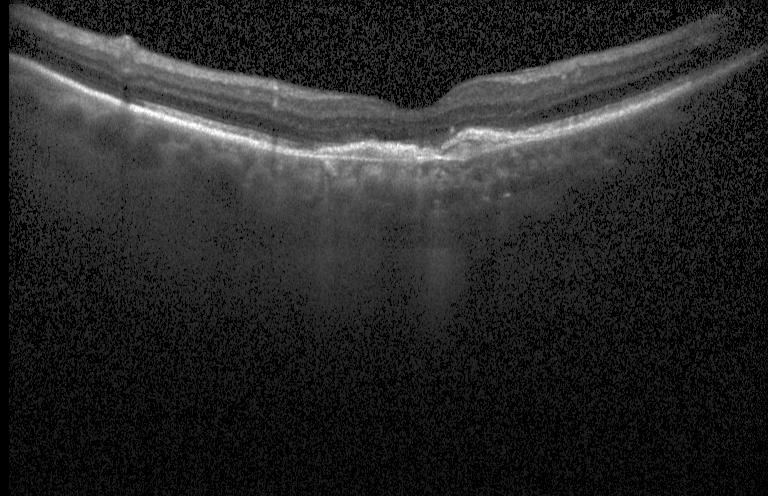 Diagnosis: a choroidal neovascular membrane.